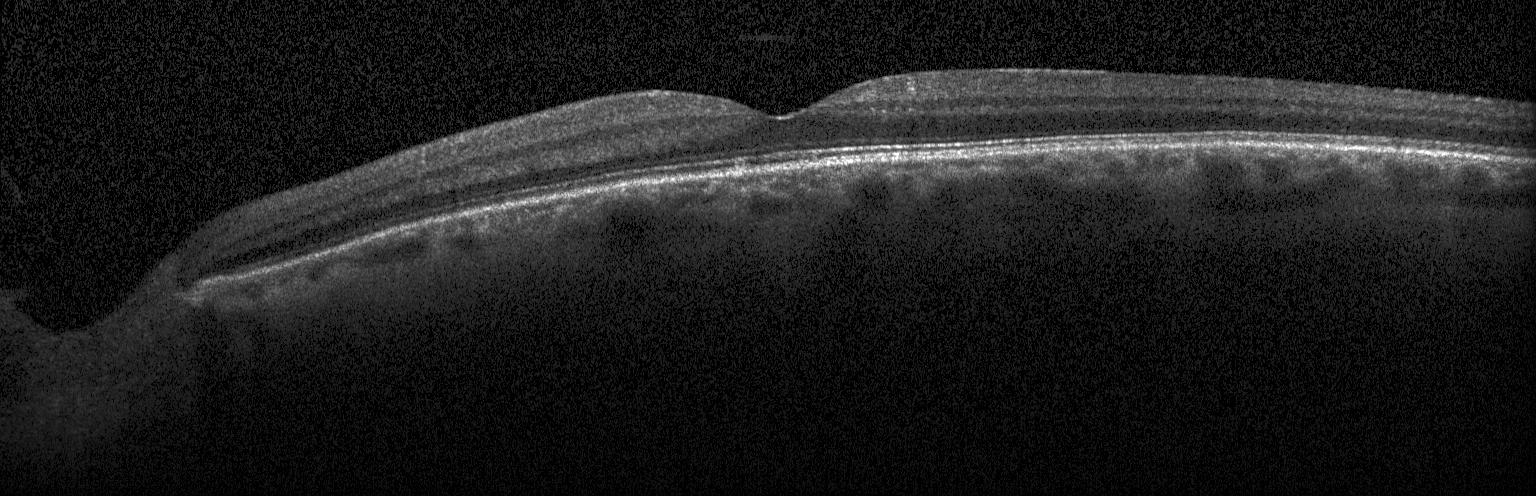

Retinal OCT cross-section showing no choroidal neovascularization, diabetic macular edema, or drusen.